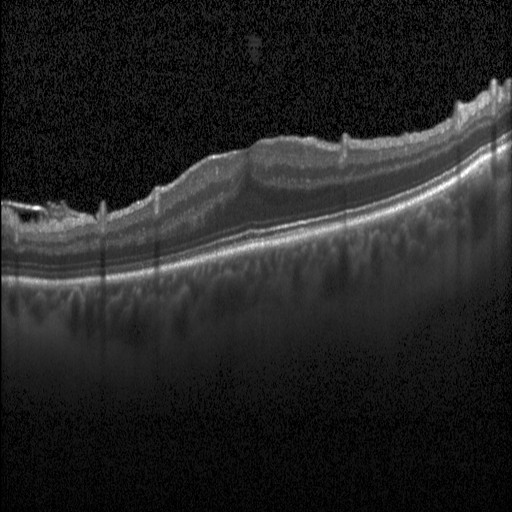 Macular OCT demonstrating diabetic macular edema (DME).